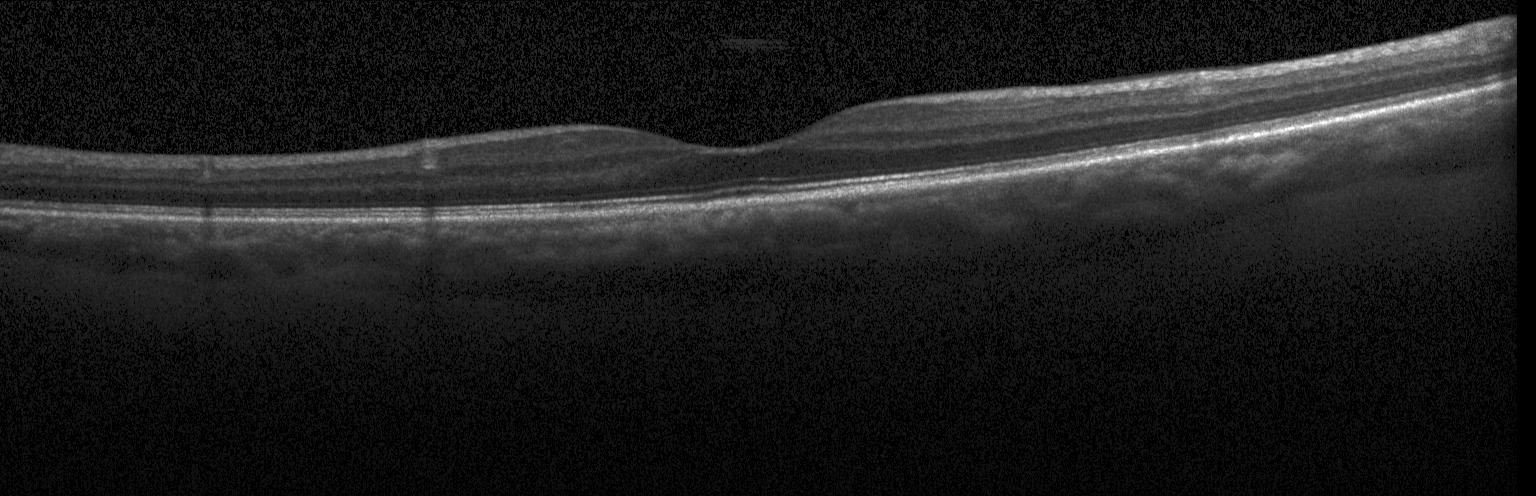
Assessment: neither CNV, DME, nor drusen.